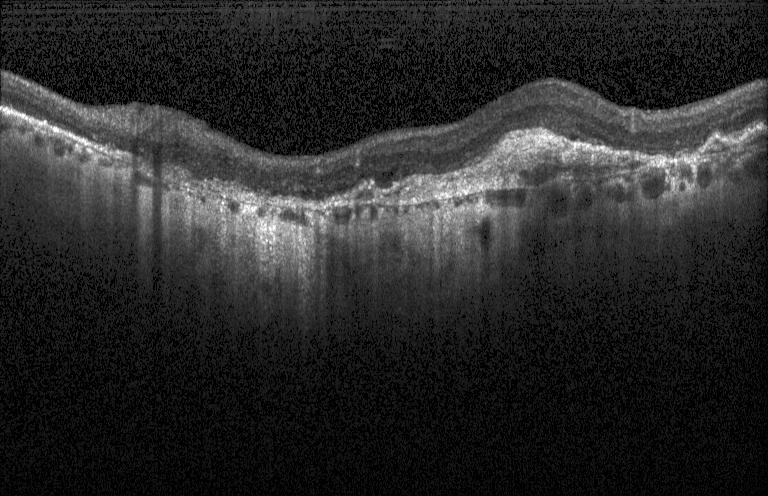
Retinal OCT cross-section
Impression: choroidal neovascularization (CNV).